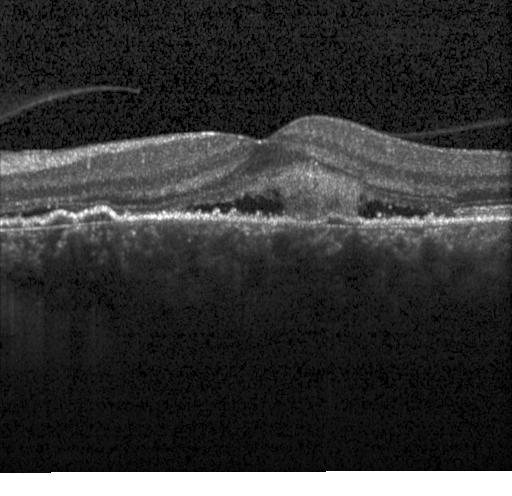

Optical coherence tomography B-scan. This B-scan demonstrates a choroidal neovascular membrane.